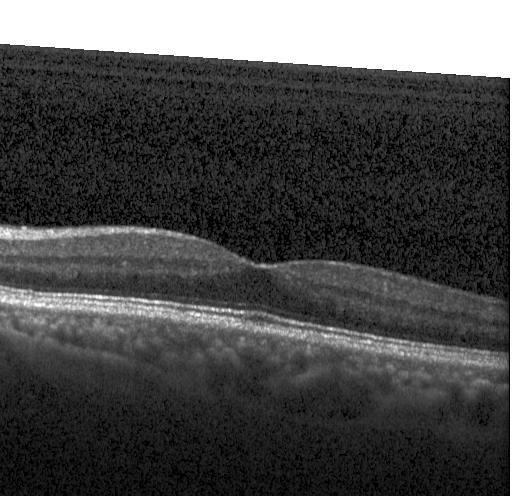
OCT B-scan · centered on the fovea · spectral-domain OCT
Diagnosis: neither choroidal neovascularization, diabetic macular edema, nor drusen.